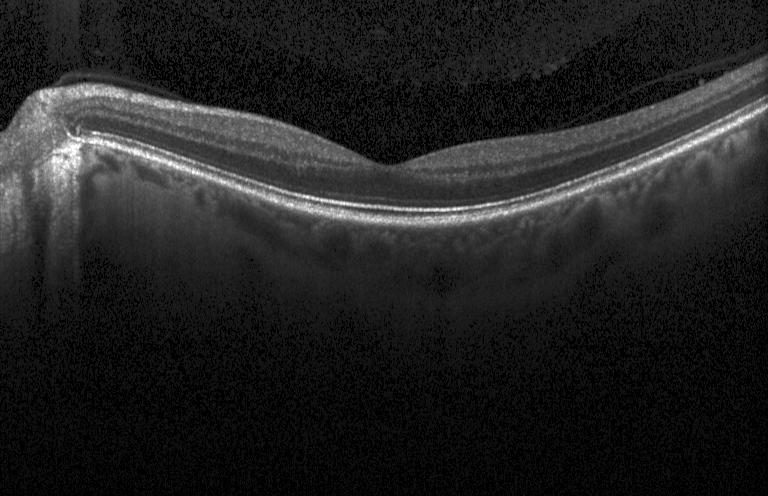
Spectral-domain OCT B-scan: no evidence of CNV, DME, or drusen.